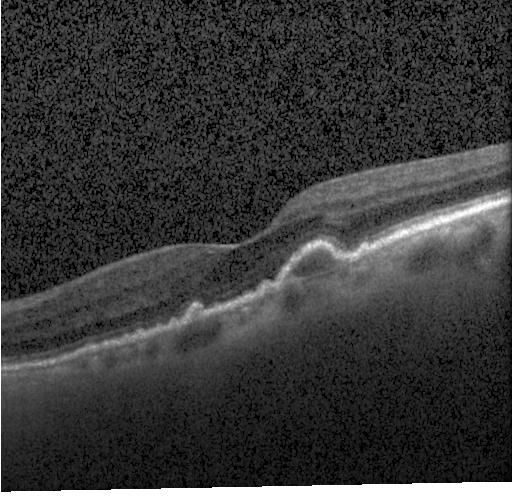 Spectral-domain OCT B-scan: choroidal neovascularization (CNV).